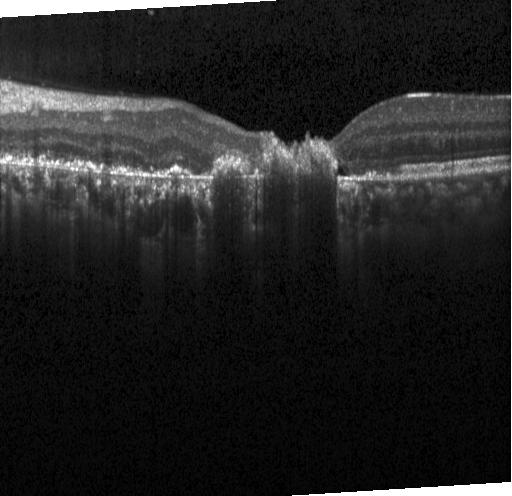

Spectral-domain optical coherence tomography; horizontal scan through the fovea; optical coherence tomography scan — Finding: a choroidal neovascular membrane.